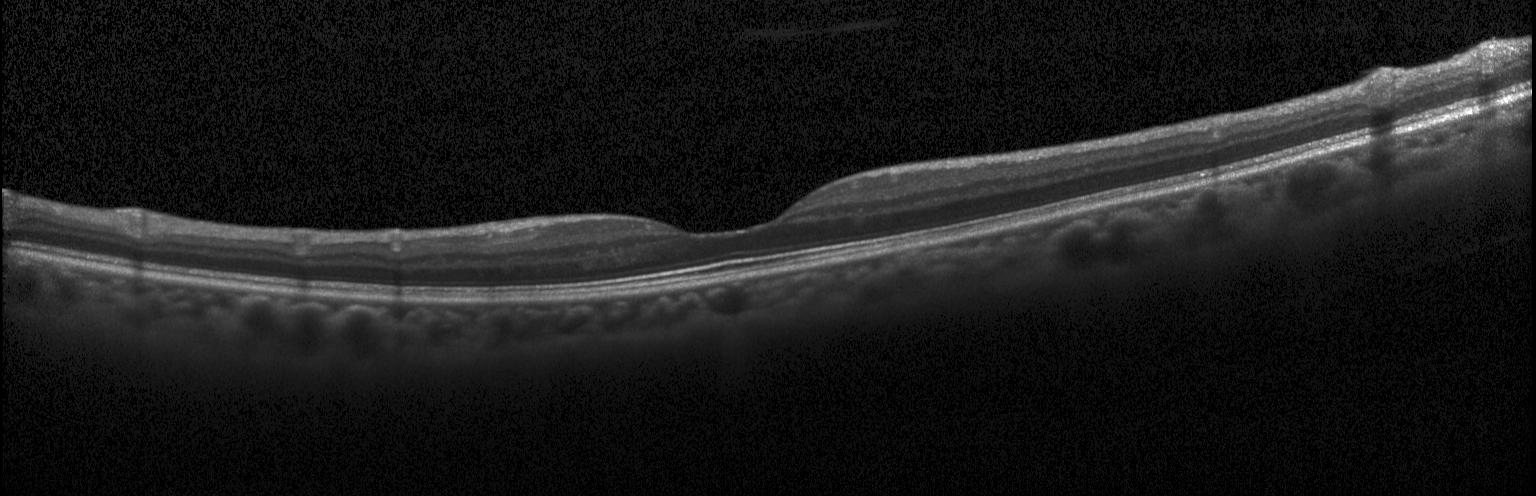 Optical coherence tomography B-scan. Assessment: no choroidal neovascularization, diabetic macular edema, or drusen.